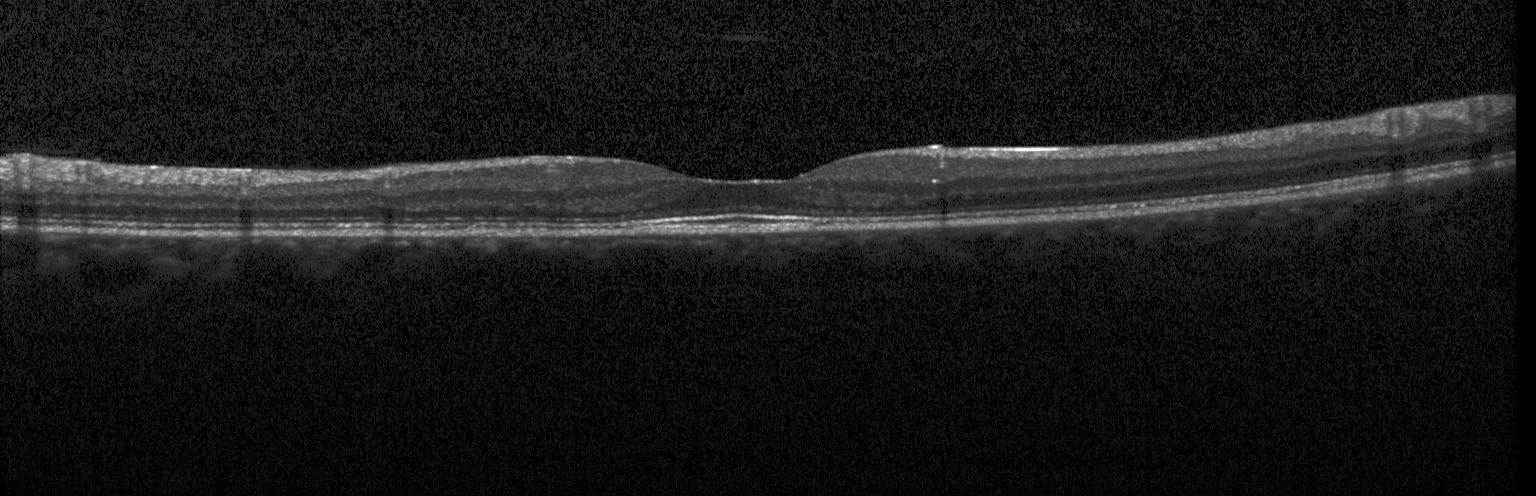

Heidelberg Spectralis · horizontal scan through the fovea · retinal OCT B-scan · spectral-domain OCT. Finding: neither CNV, DME, nor drusen.